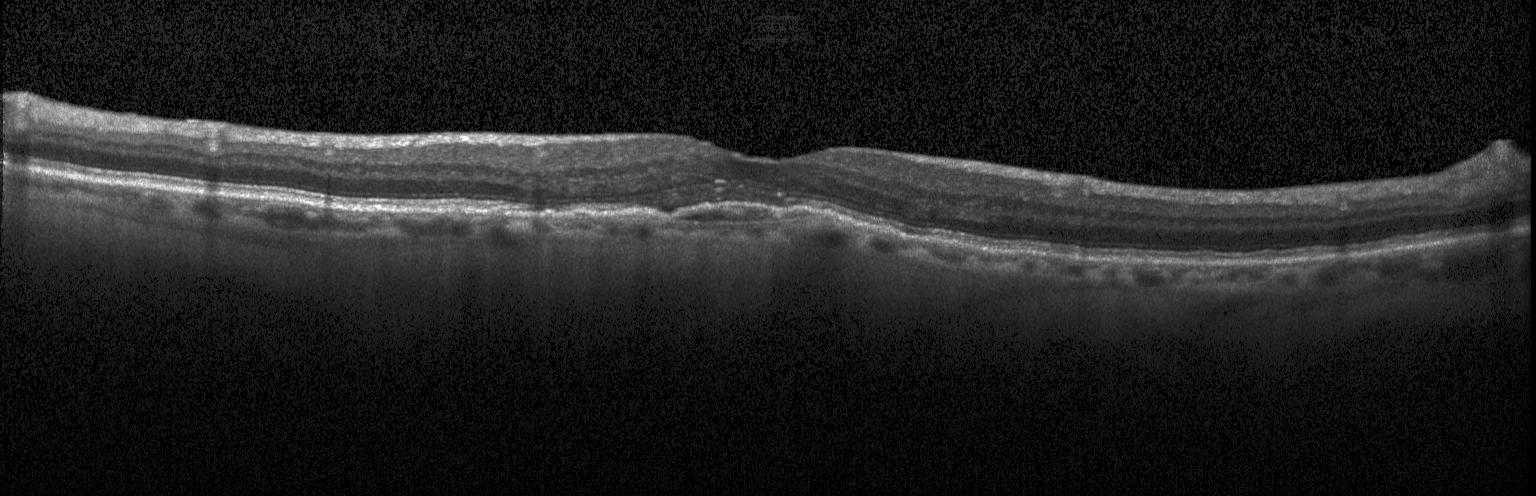

OCT line scan · fovea-centered. Assessment: a choroidal neovascular membrane.